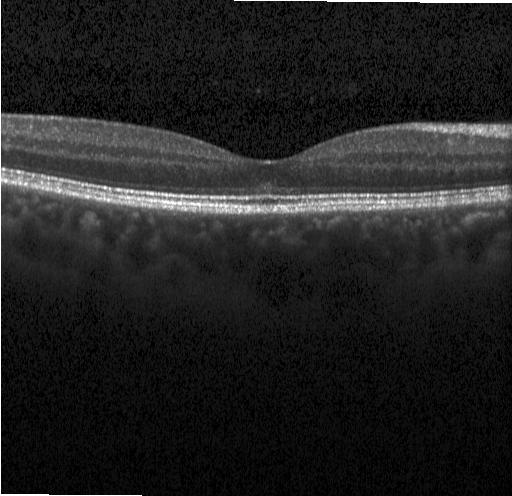

OCT finding: no choroidal neovascularization, no diabetic macular edema, and no drusen.